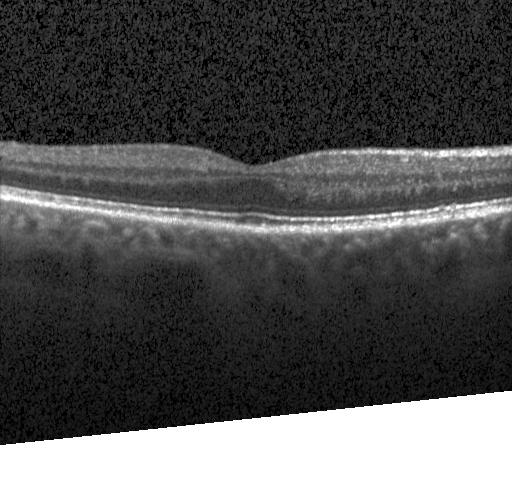 Heidelberg Spectralis OCT system · retinal OCT cross-section · SD-OCT · horizontal scan through the fovea. Dx: no evidence of choroidal neovascularization, diabetic macular edema, or drusen.